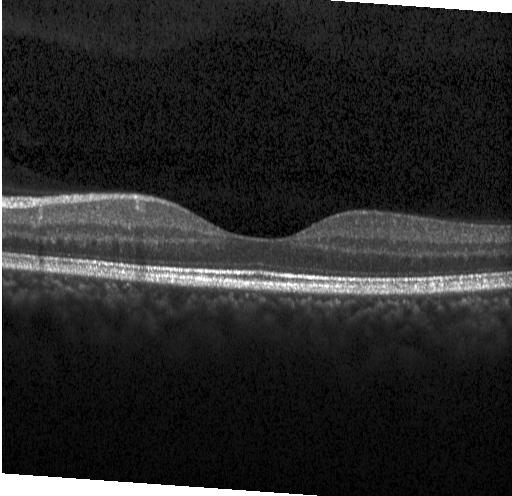

Through the macula; OCT B-scan; spectral-domain optical coherence tomography
Dx: no CNV, DME, or drusen.